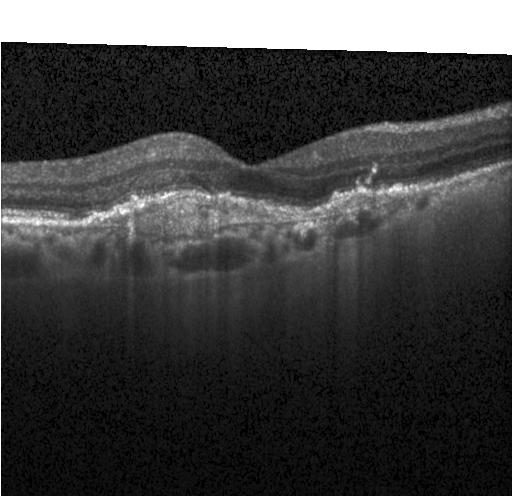
OCT line scan. Heidelberg Spectralis. Macular scan. Spectral-domain OCT.
Diagnosis: a choroidal neovascular membrane.